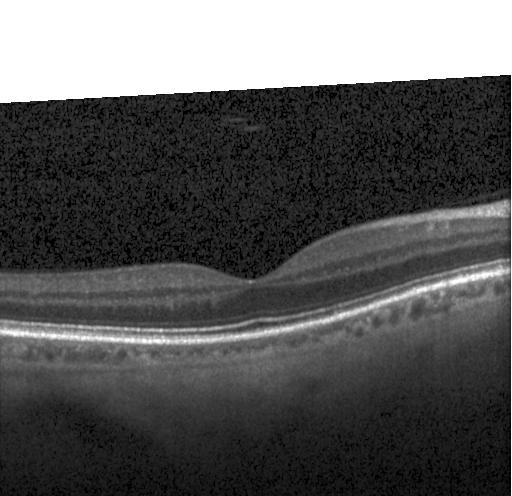

SD-OCT · retinal OCT B-scan.
Neither choroidal neovascularization, diabetic macular edema, nor drusen.